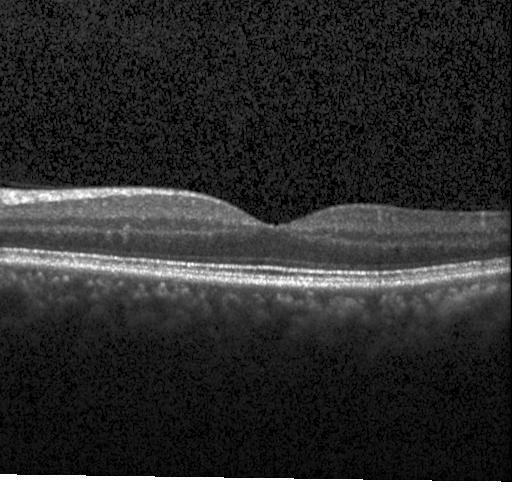
OCT line scan. No evidence of choroidal neovascularization, diabetic macular edema, or drusen.